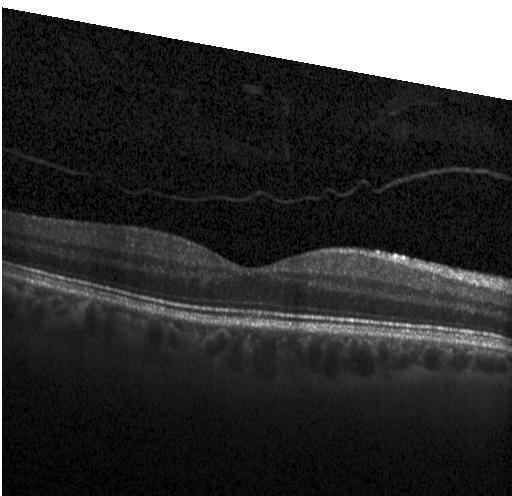

Macular OCT demonstrating neither choroidal neovascularization, diabetic macular edema, nor drusen.